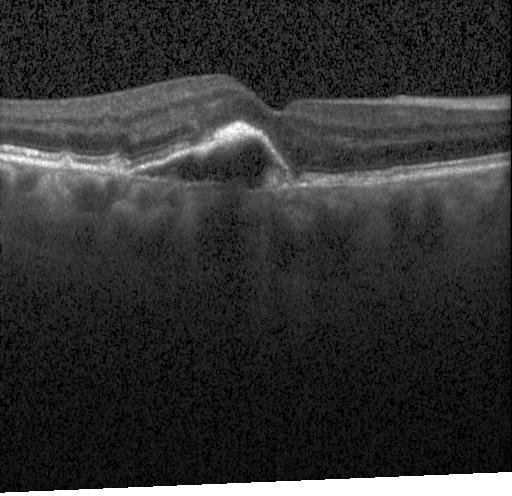

Horizontal scan through the fovea, retinal OCT cross-section. Choroidal neovascularization (CNV).